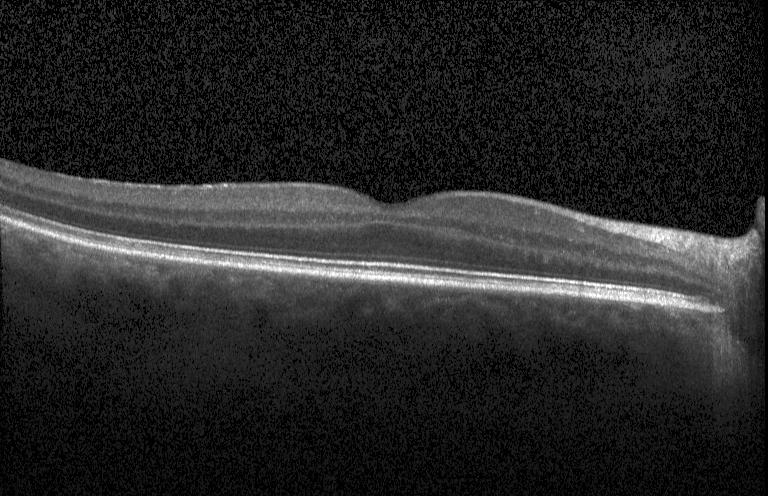 Impression: no choroidal neovascularization, diabetic macular edema, or drusen.